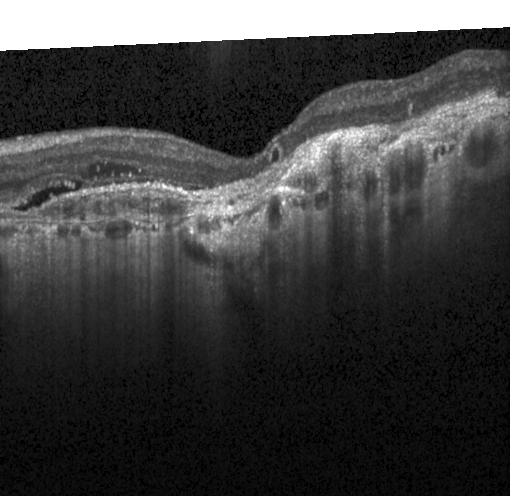

The scan shows a choroidal neovascular membrane.